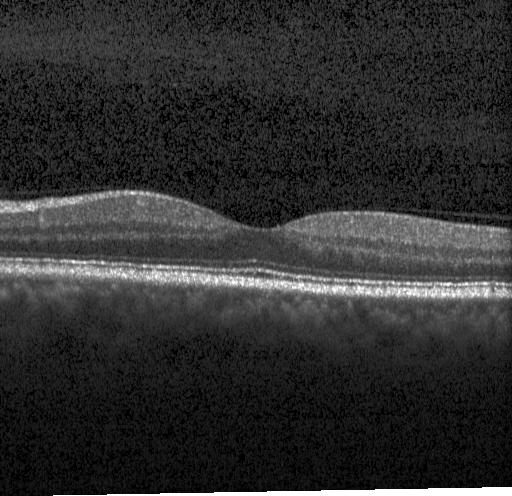
Through the macula; retinal OCT B-scan. Dx: no evidence of choroidal neovascularization, diabetic macular edema, or drusen.